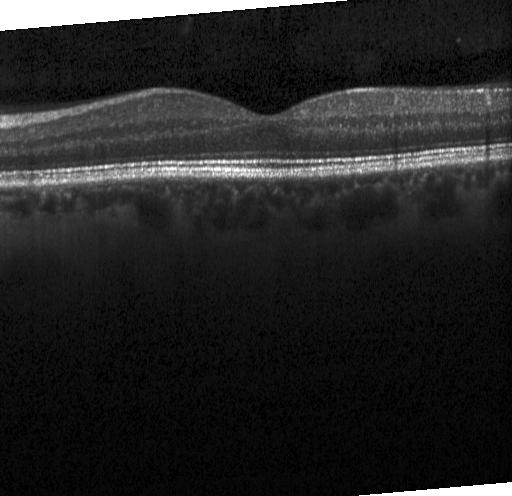 Retinal OCT cross-section. This B-scan demonstrates no evidence of choroidal neovascularization, diabetic macular edema, or drusen.